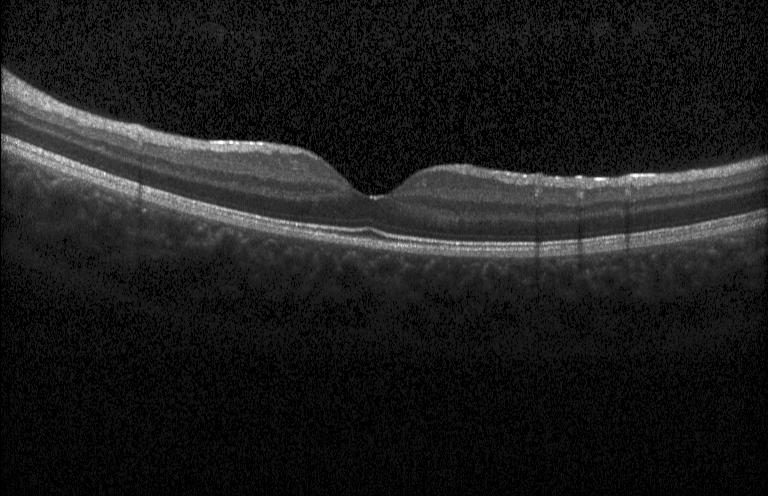
This B-scan demonstrates no evidence of choroidal neovascularization, diabetic macular edema, or drusen.